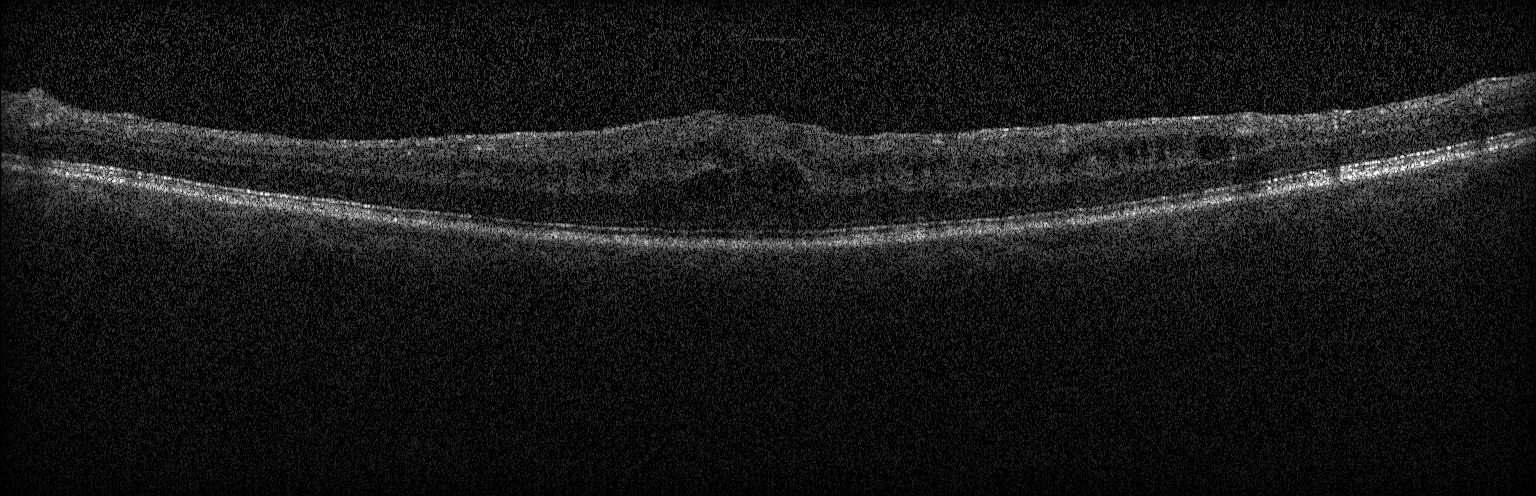
Optical coherence tomography B-scan — Diagnosis: diabetic macular edema (DME).